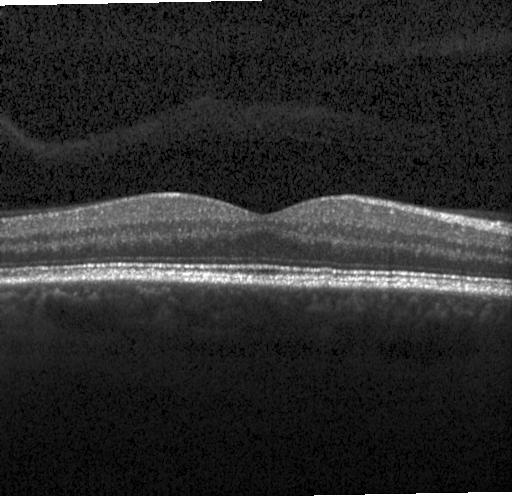

Centered on the fovea; optical coherence tomography scan; spectral-domain optical coherence tomography. Finding: neither choroidal neovascularization, diabetic macular edema, nor drusen.